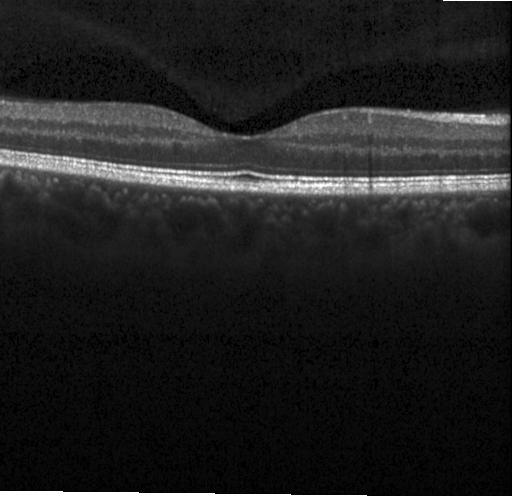 Horizontal scan through the fovea; Heidelberg Spectralis; OCT line scan. This B-scan demonstrates no evidence of choroidal neovascularization, diabetic macular edema, or drusen.